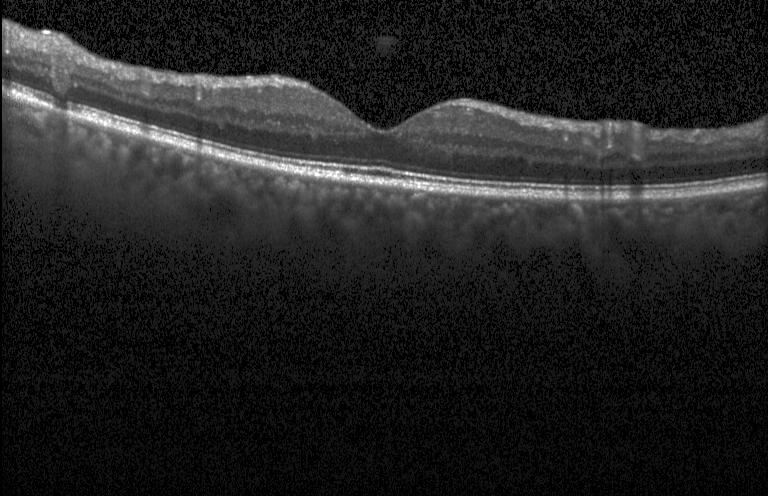 Spectral-domain optical coherence tomography, centered on the fovea, Heidelberg Spectralis OCT system, optical coherence tomography scan
This B-scan demonstrates no CNV, DME, or drusen.